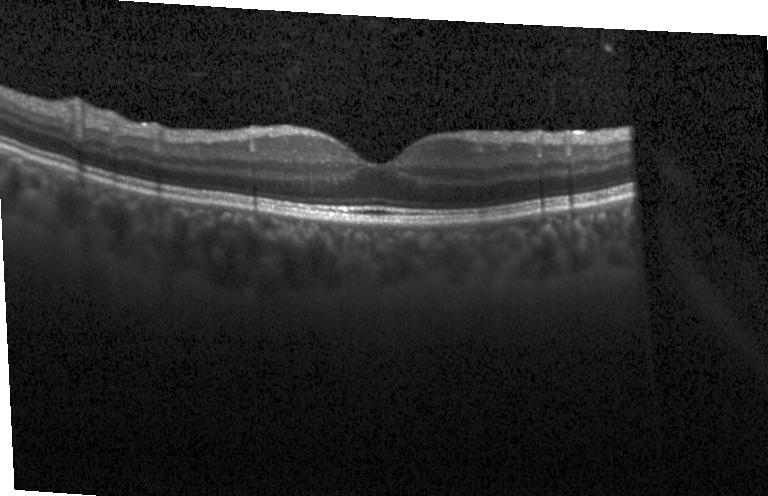

Macular OCT demonstrating neither CNV, DME, nor drusen.